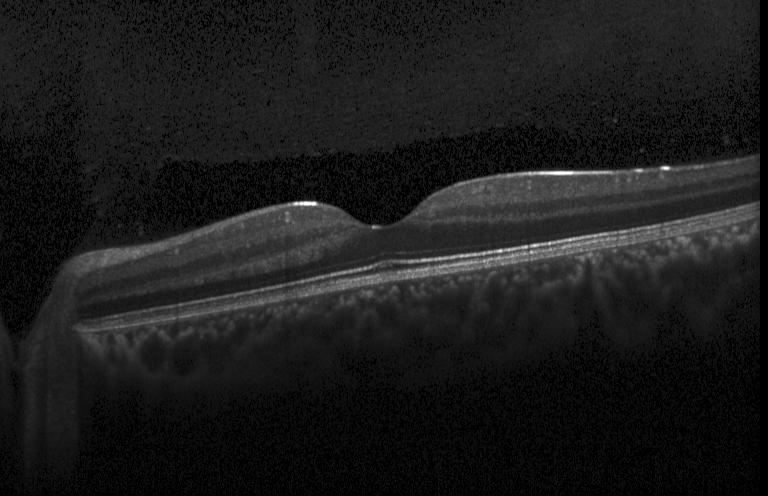 OCT scan showing no choroidal neovascularization, no diabetic macular edema, and no drusen.